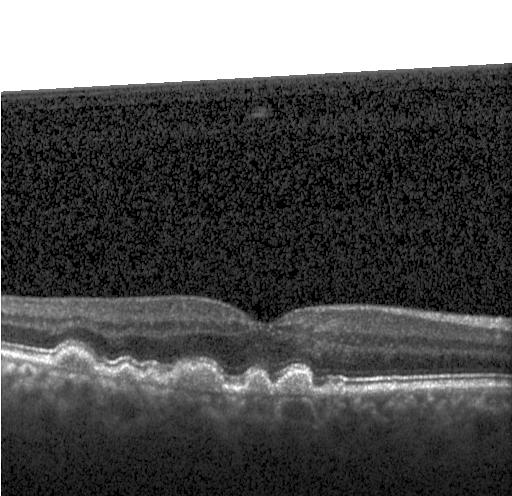
OCT B-scan showing drusen.